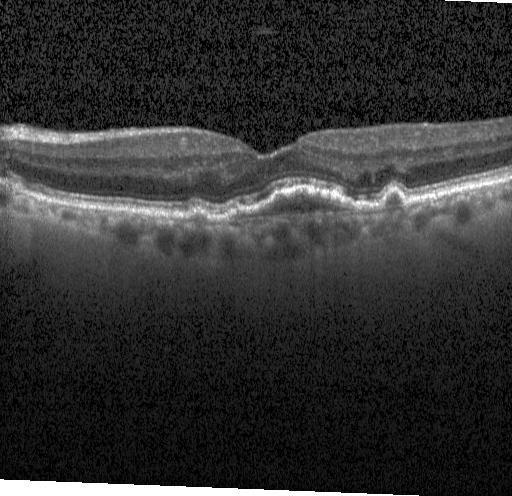 Horizontal scan through the fovea. Spectral-domain optical coherence tomography. Instrument: Heidelberg Spectralis. OCT B-scan.
The scan shows a choroidal neovascular membrane.